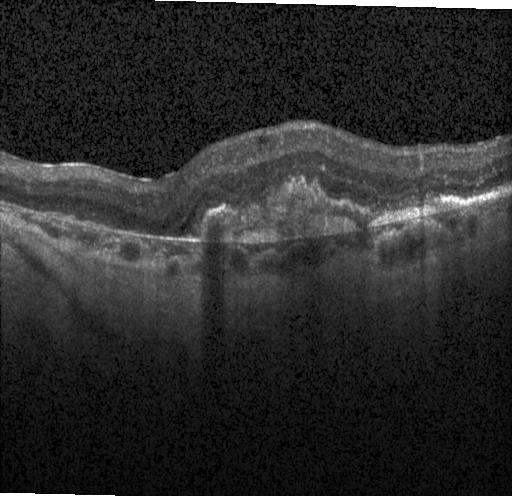
Impression: choroidal neovascularization (CNV).